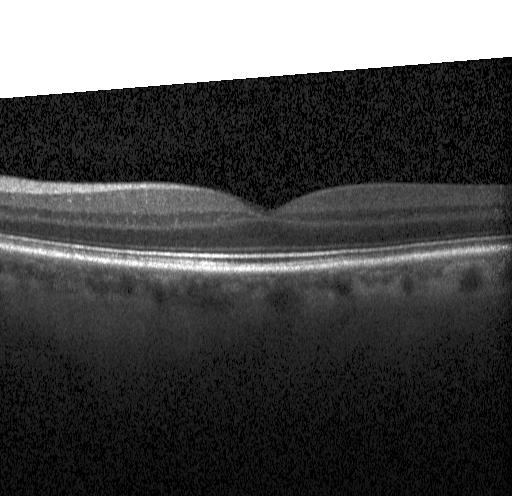

Finding: neither choroidal neovascularization, diabetic macular edema, nor drusen.